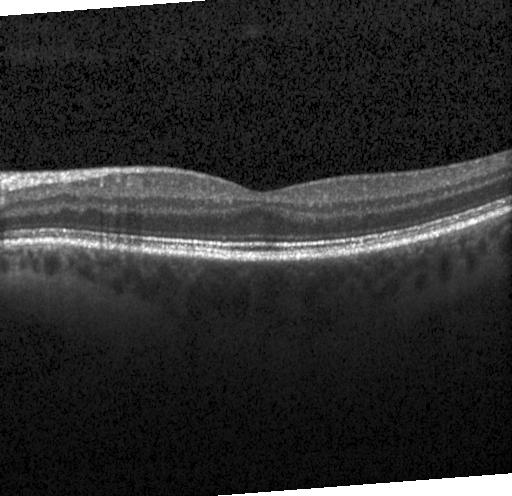 Diagnosis: neither CNV, DME, nor drusen.